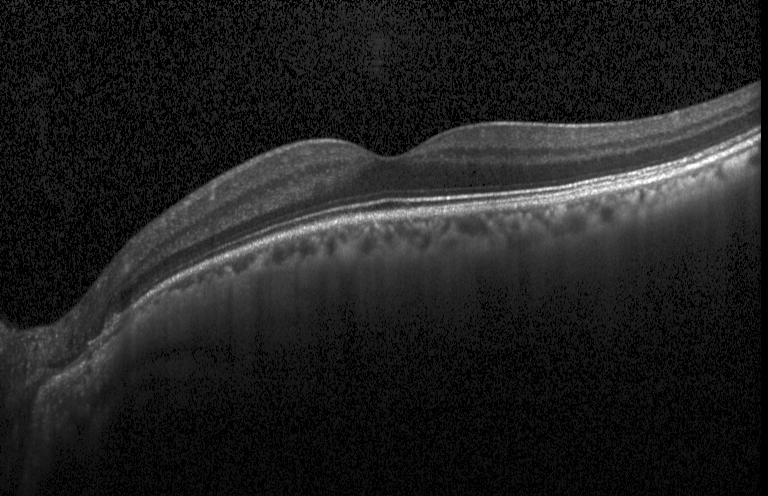

Assessment: neither CNV, DME, nor drusen.